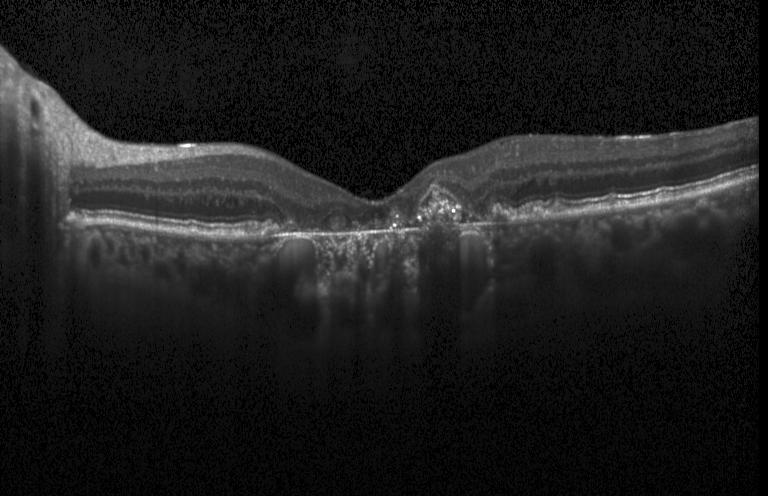 Dx: choroidal neovascularization (CNV).